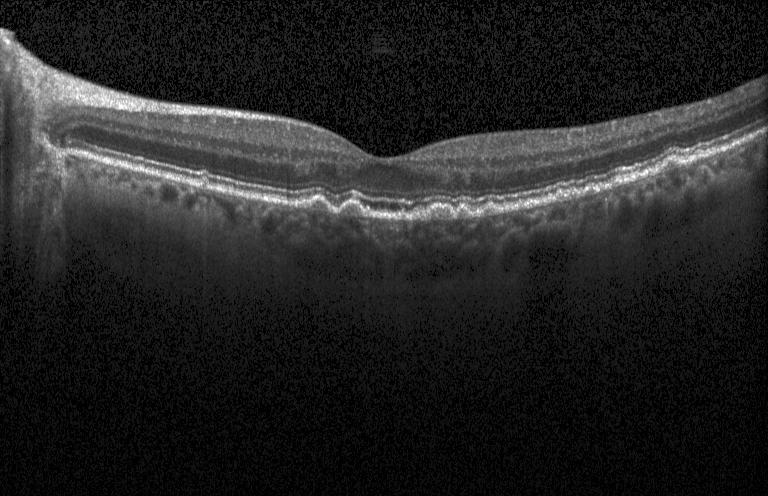

Optical coherence tomography B-scan.
Impression: drusen.